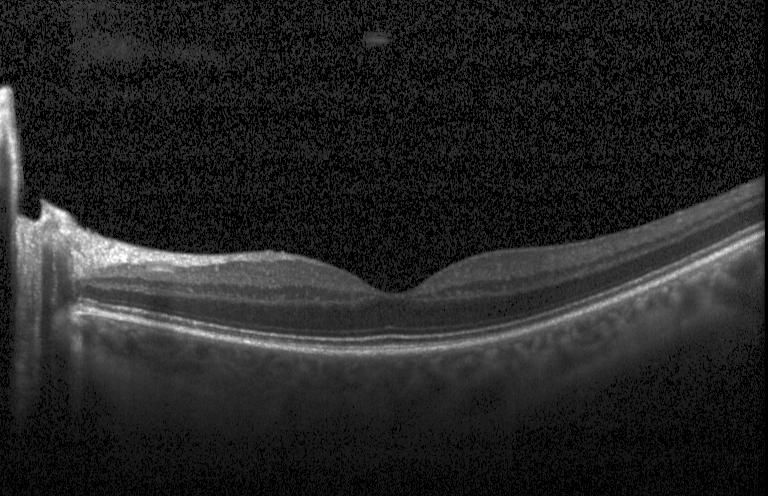

OCT B-scan, SD-OCT, macular scan
OCT finding: neither choroidal neovascularization, diabetic macular edema, nor drusen.